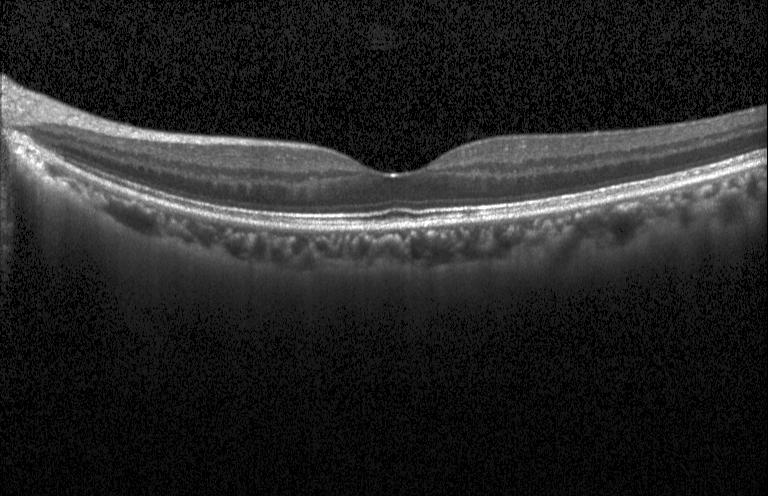
Optical coherence tomography scan · Heidelberg Spectralis OCT system.
This B-scan demonstrates neither choroidal neovascularization, diabetic macular edema, nor drusen.